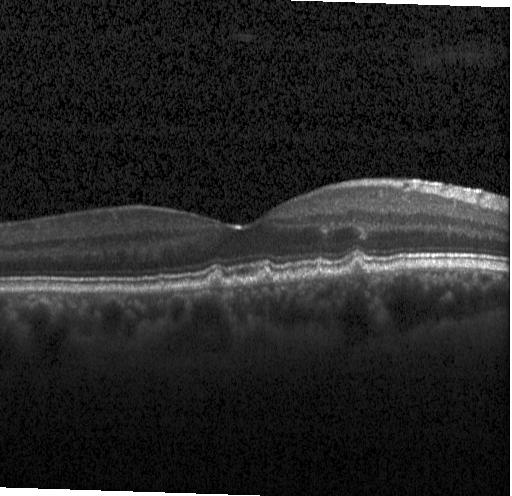

OCT B-scan
OCT finding: multiple drusen.